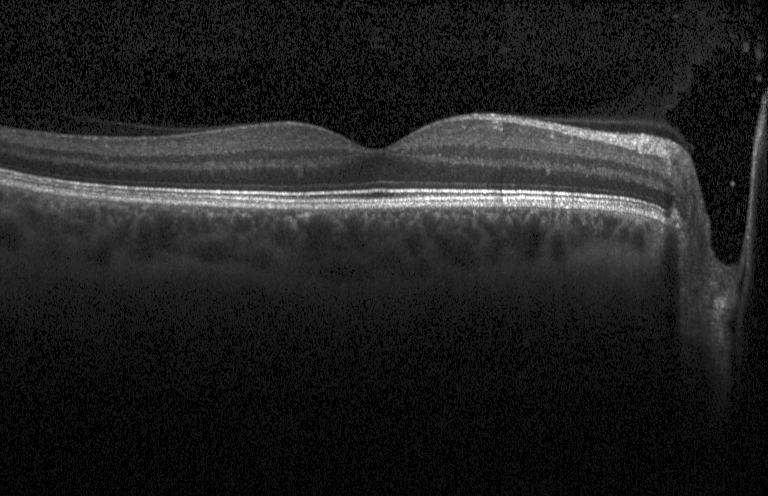 Optical coherence tomography scan · SD-OCT — OCT finding: no evidence of CNV, DME, or drusen.